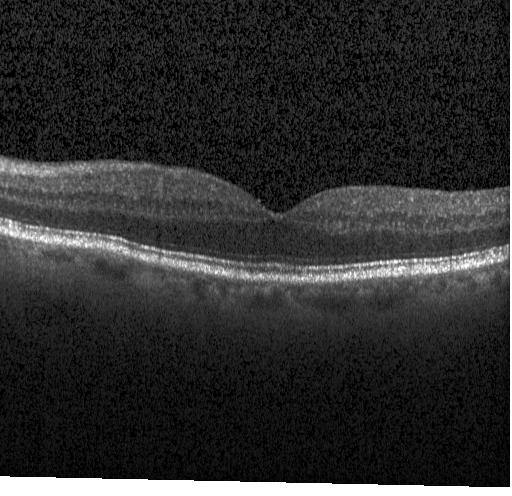 Through the macula · retinal OCT B-scan.
Diagnosis: no evidence of CNV, DME, or drusen.